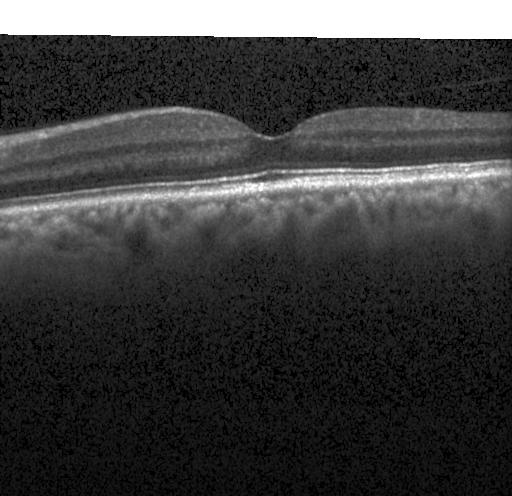 Assessment: no choroidal neovascularization, diabetic macular edema, or drusen.